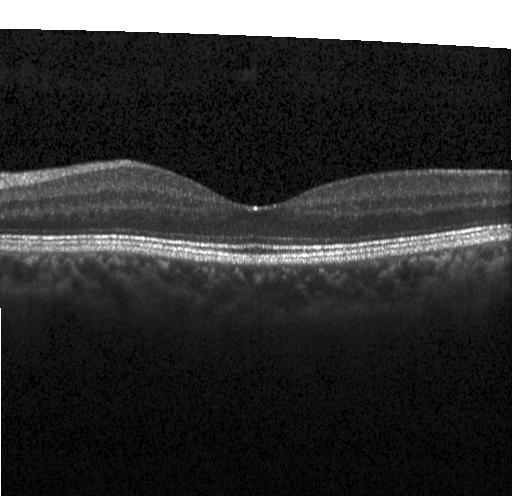
Optical coherence tomography B-scan — Impression: neither choroidal neovascularization, diabetic macular edema, nor drusen.